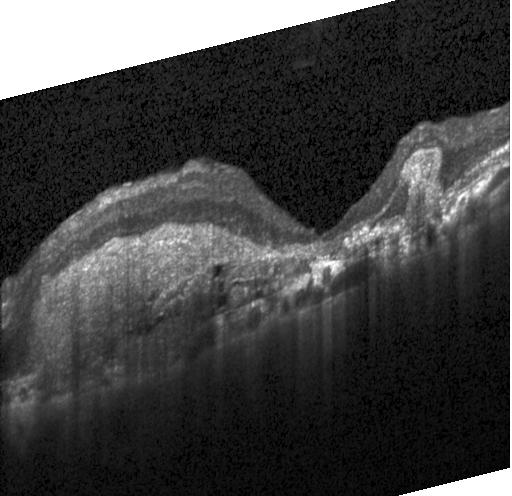
Assessment: CNV.